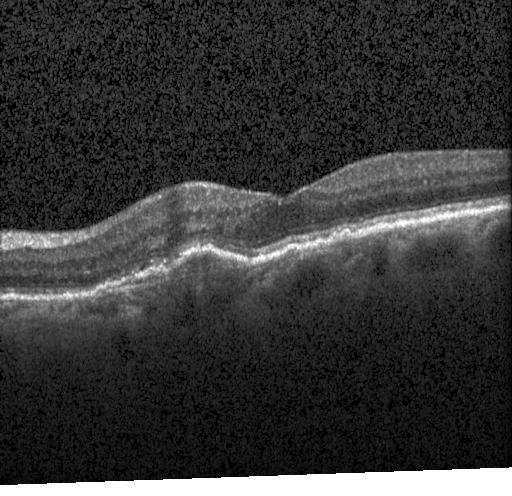
Instrument: Heidelberg Spectralis · OCT line scan · through the macula.
This B-scan demonstrates CNV.